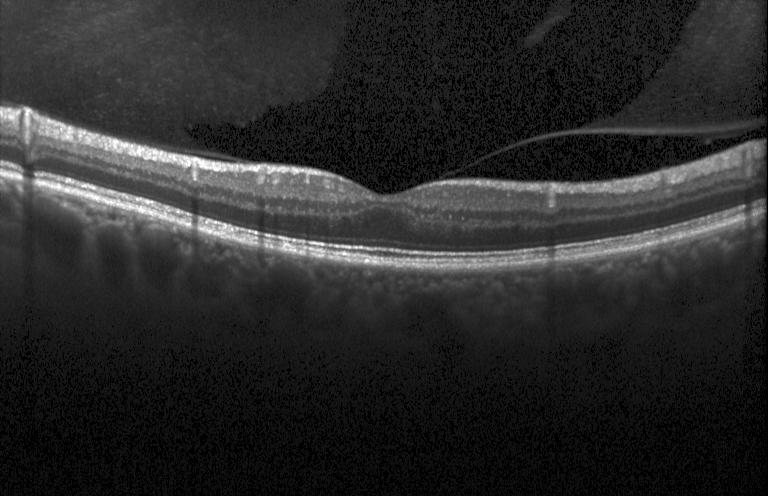
Retinal OCT B-scan. Diagnosis: no choroidal neovascularization, no diabetic macular edema, and no drusen.